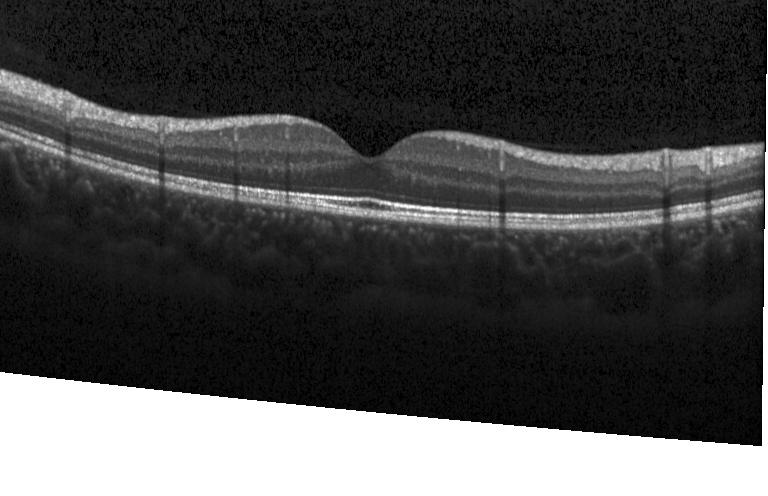 Retinal OCT B-scan; centered on the fovea; Heidelberg Spectralis OCT system; spectral-domain optical coherence tomography.
Finding: no choroidal neovascularization, diabetic macular edema, or drusen.